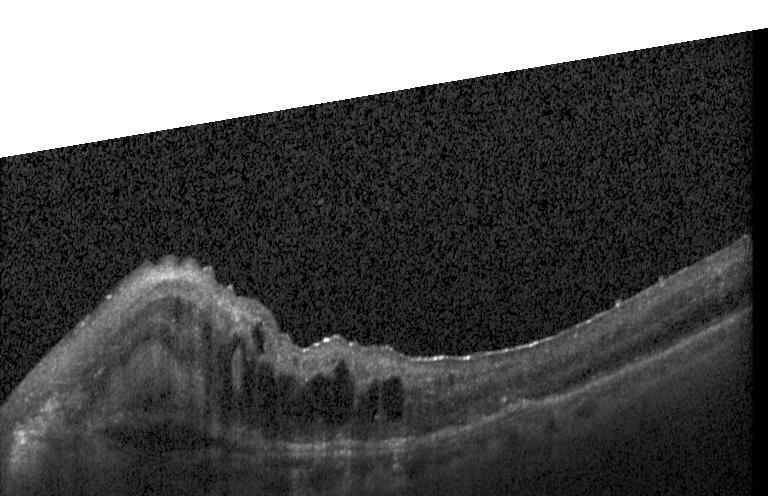

OCT line scan. Finding: CNV.